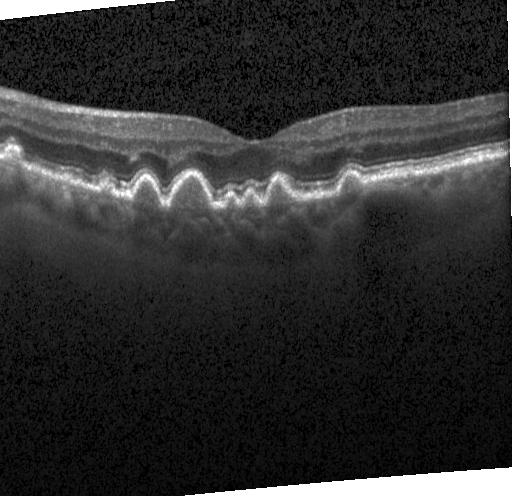
Impression: multiple drusen.